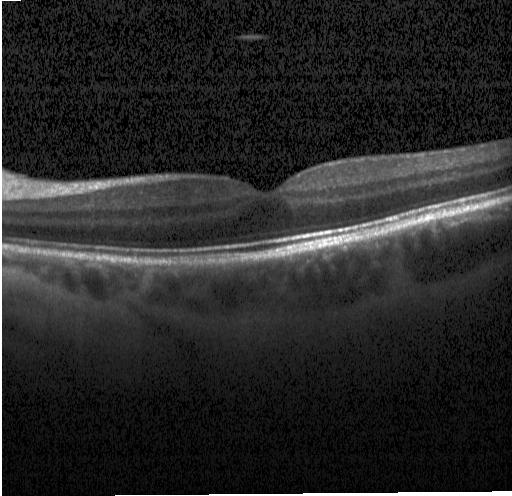
Fovea-centered; optical coherence tomography scan. Finding: no evidence of choroidal neovascularization, diabetic macular edema, or drusen.